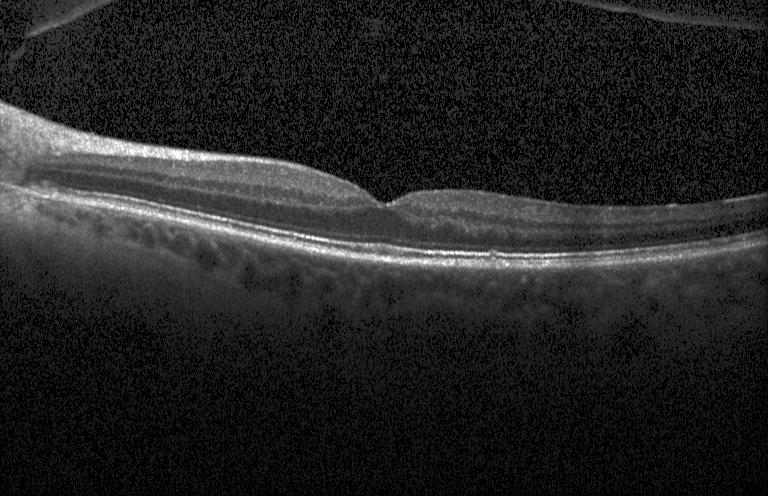
OCT B-scan; spectral-domain optical coherence tomography; instrument: Heidelberg Spectralis — Multiple drusen.